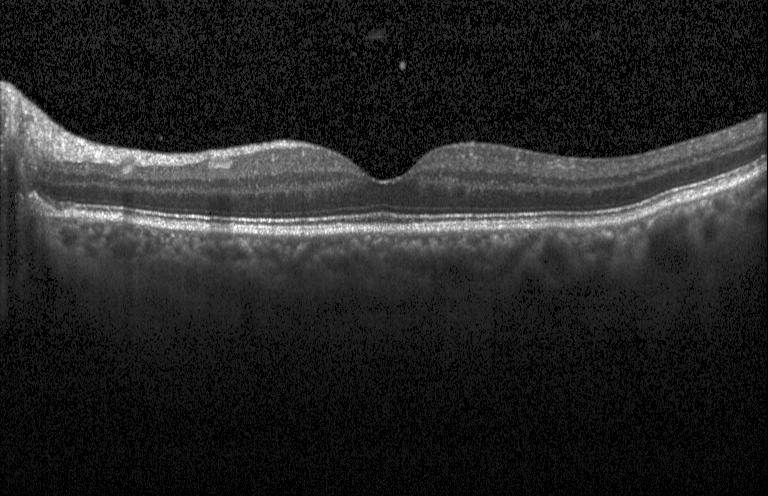

OCT line scan
OCT finding: neither CNV, DME, nor drusen.